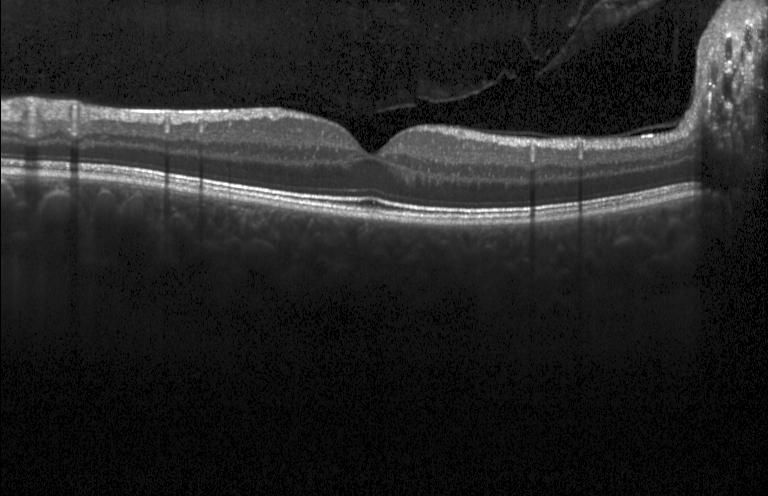 Finding: no evidence of choroidal neovascularization, diabetic macular edema, or drusen.